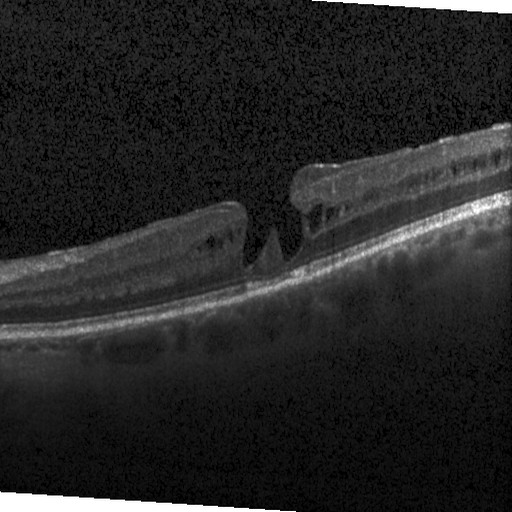

Retinal OCT cross-section showing DME.